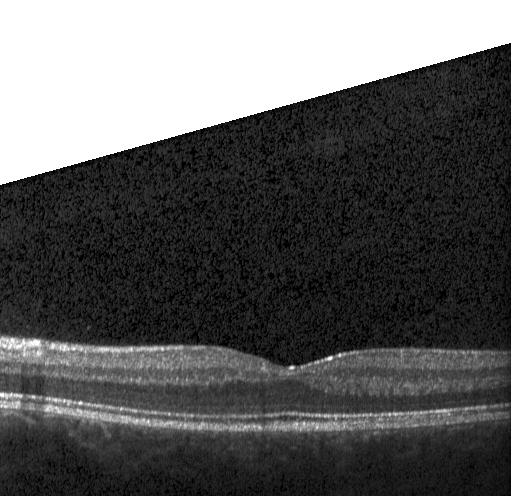 Macular OCT: no CNV, DME, or drusen.